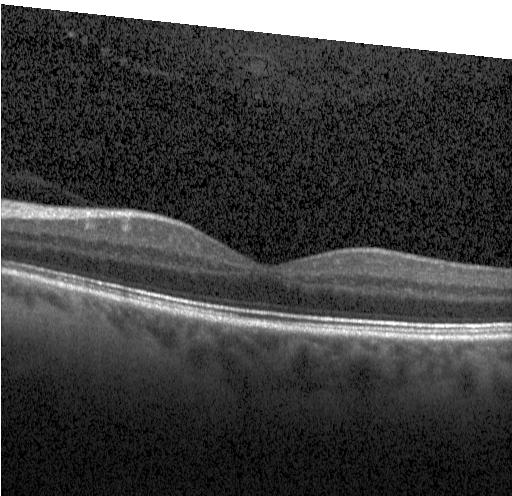 Retinal OCT cross-section; instrument: Heidelberg Spectralis; SD-OCT; macular scan. OCT finding: no CNV, DME, or drusen.